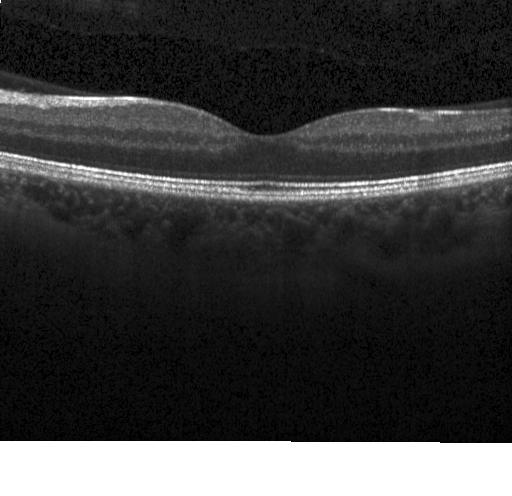

Centered on the fovea · optical coherence tomography scan · Heidelberg Spectralis OCT system. Finding: no CNV, DME, or drusen.